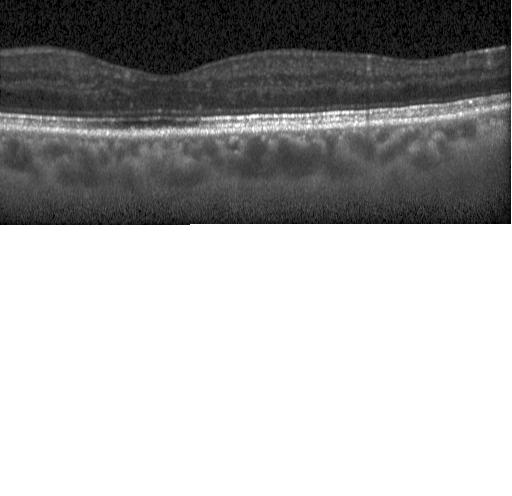 OCT B-scan showing neither choroidal neovascularization, diabetic macular edema, nor drusen.